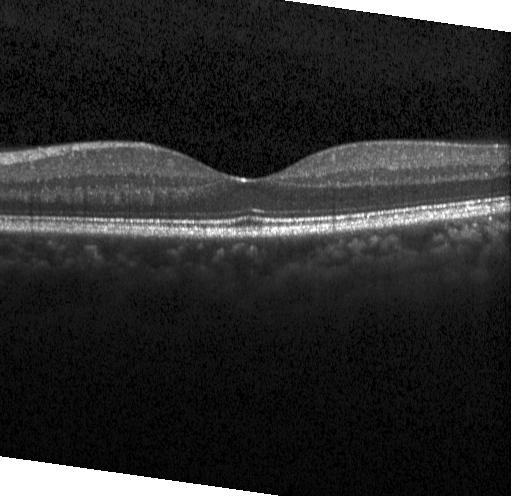
OCT finding: no CNV, no DME, and no drusen.